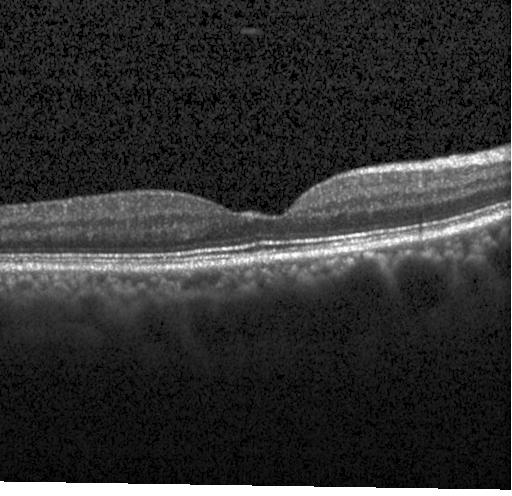
OCT line scan. Impression: neither choroidal neovascularization, diabetic macular edema, nor drusen.